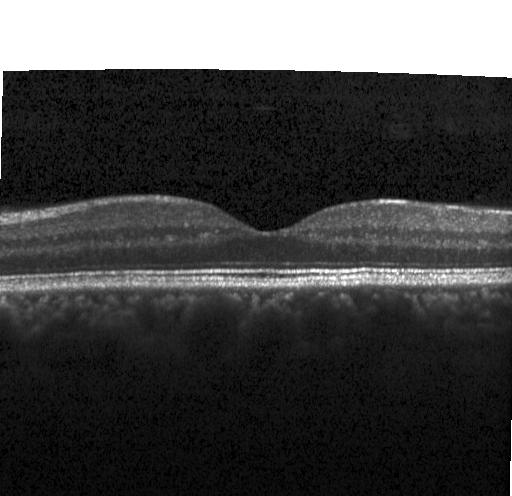
Macular OCT demonstrating no evidence of CNV, DME, or drusen.